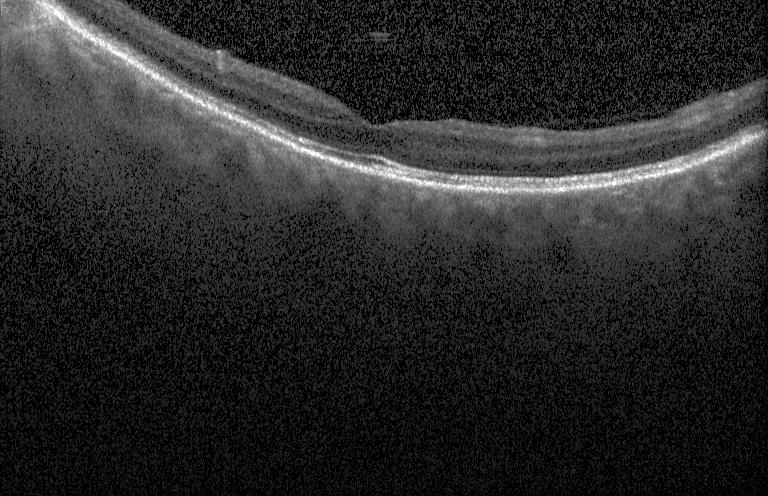
Heidelberg Spectralis OCT system; spectral-domain optical coherence tomography; OCT line scan — The scan shows no evidence of CNV, DME, or drusen.